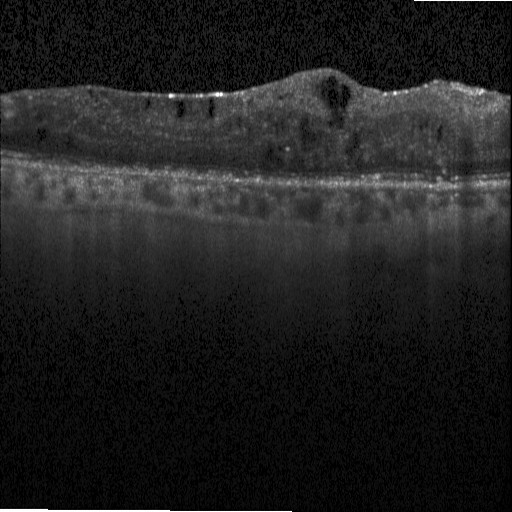 Retinal OCT cross-section. Diabetic macular edema.